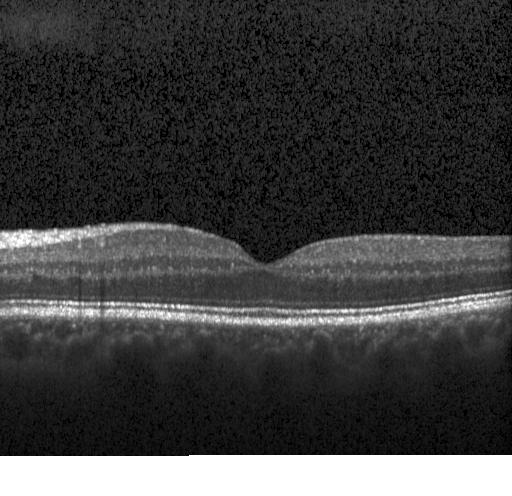
Optical coherence tomography scan.
Finding: neither choroidal neovascularization, diabetic macular edema, nor drusen.